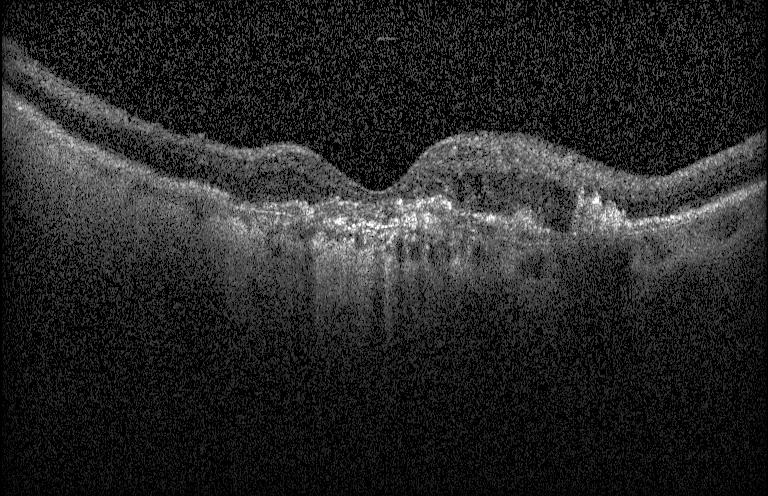

SD-OCT · Heidelberg Spectralis OCT system · retinal OCT cross-section · centered on the fovea — Impression: a choroidal neovascular membrane.